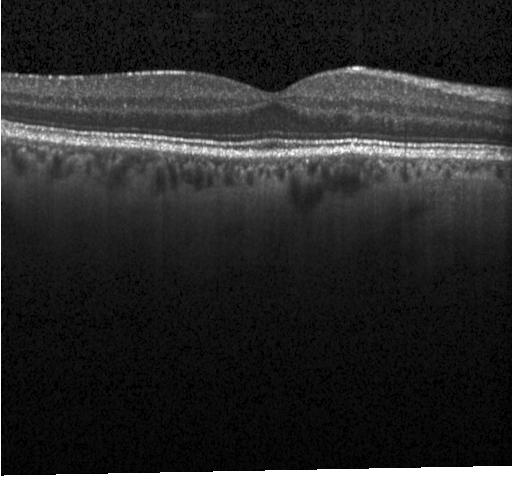 OCT line scan.
Diagnosis: neither choroidal neovascularization, diabetic macular edema, nor drusen.